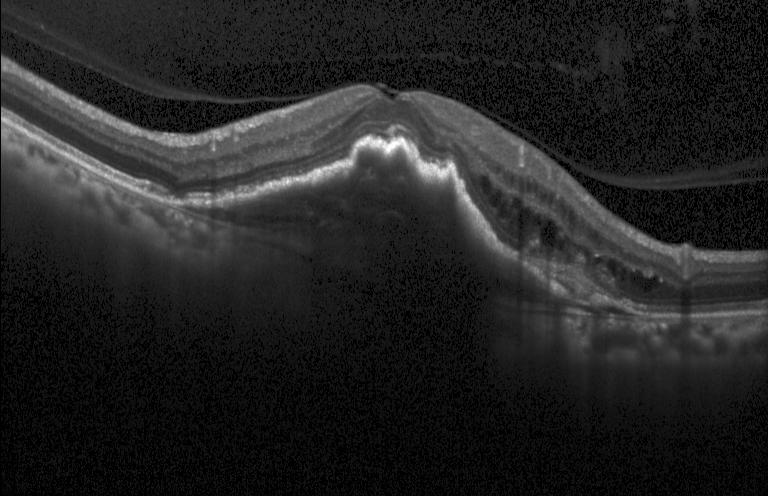

Optical coherence tomography scan · Heidelberg Spectralis OCT system
Dx: choroidal neovascularization (CNV).